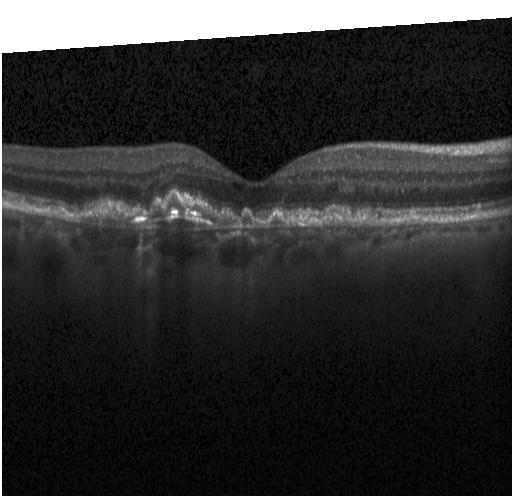

OCT B-scan showing a choroidal neovascular membrane.